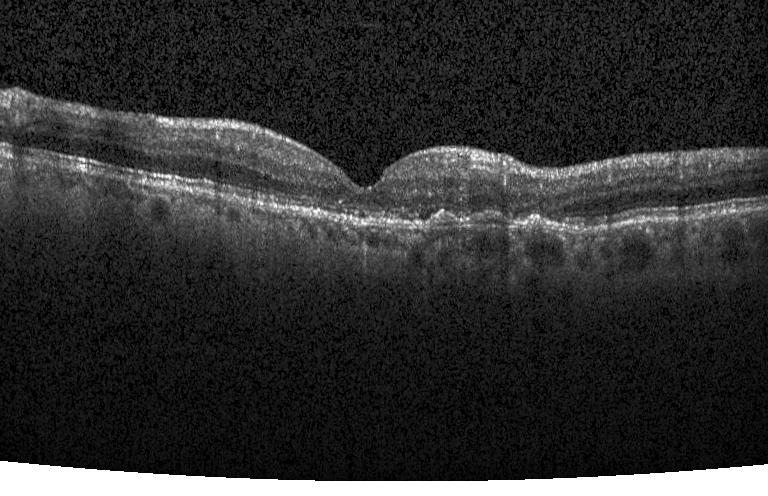 Retinal OCT B-scan · instrument: Heidelberg Spectralis. Dx: a choroidal neovascular membrane.